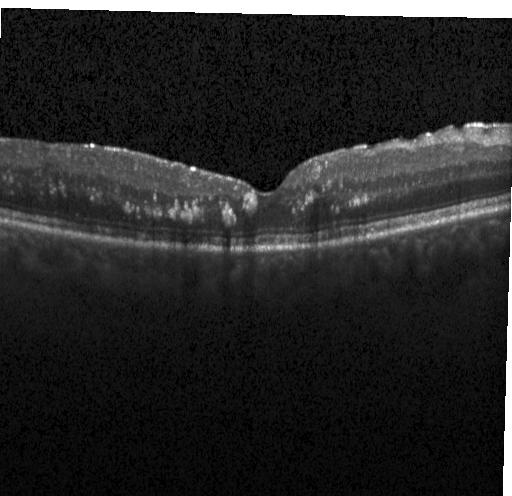
Impression: diabetic macular edema.